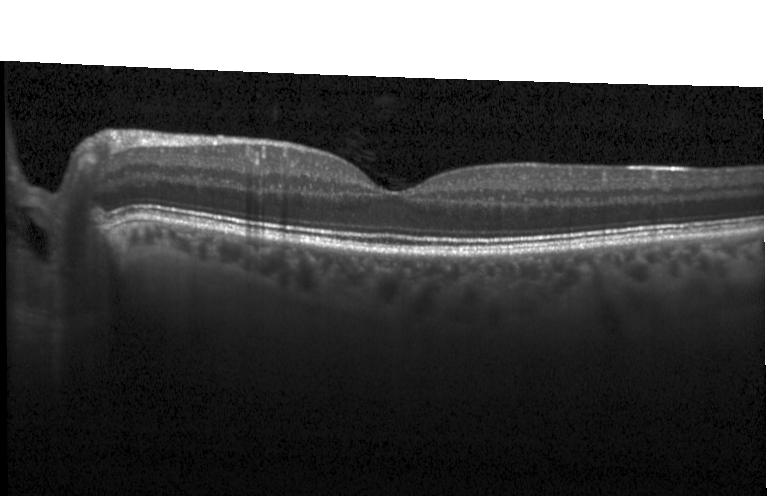

OCT finding: no CNV, no DME, and no drusen.